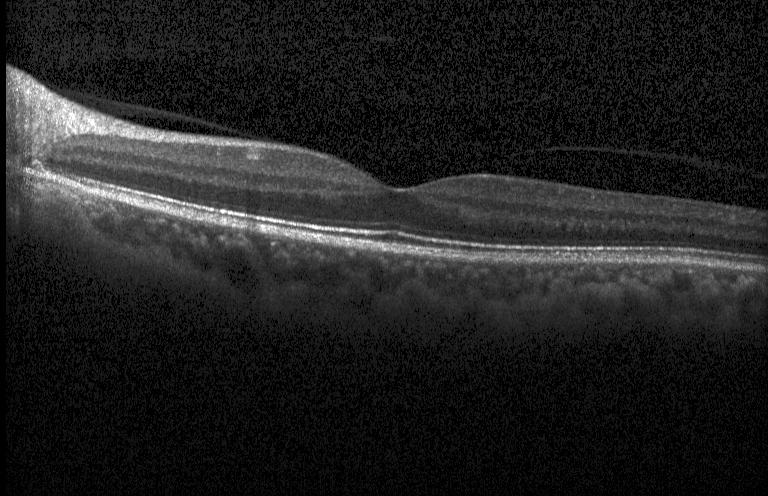

Retinal OCT B-scan.
OCT finding: no evidence of CNV, DME, or drusen.